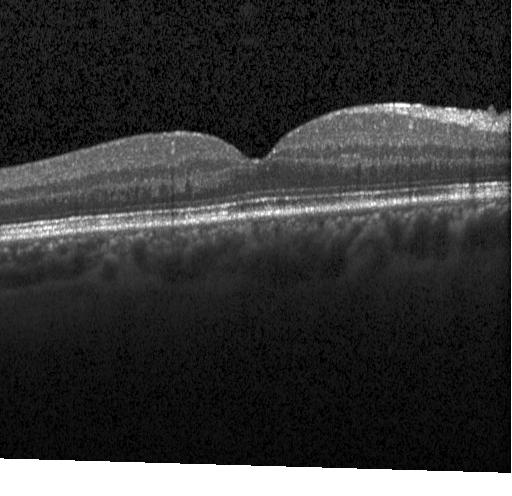
Finding: neither choroidal neovascularization, diabetic macular edema, nor drusen.